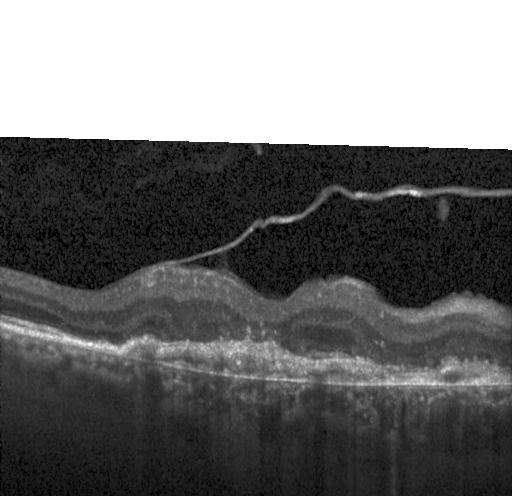
OCT finding: CNV.